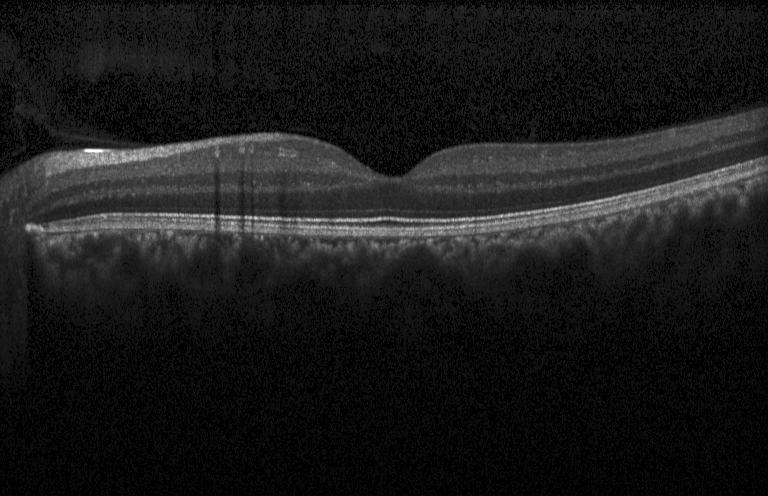

Optical coherence tomography scan.
Impression: neither CNV, DME, nor drusen.